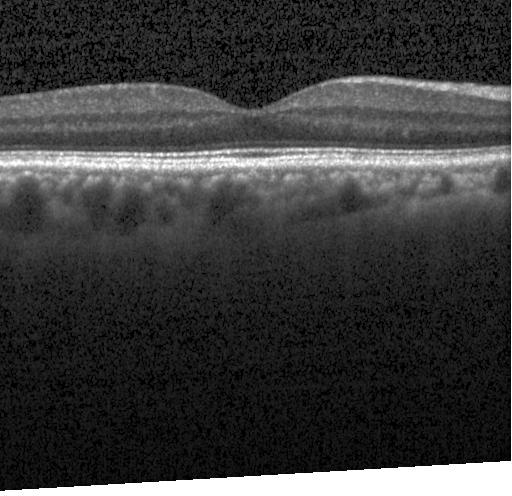
Spectral-domain OCT B-scan: no evidence of choroidal neovascularization, diabetic macular edema, or drusen.